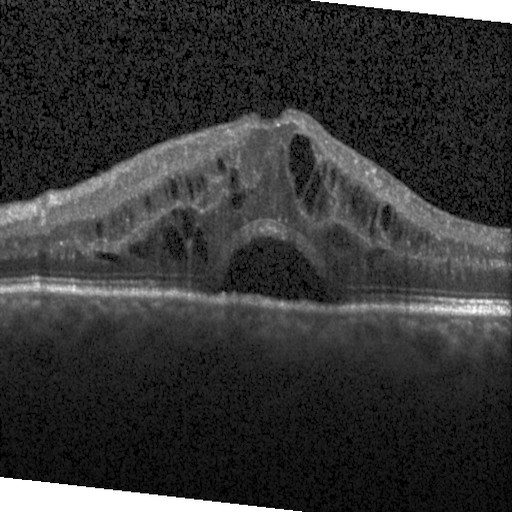
Spectral-domain OCT; OCT B-scan
This B-scan demonstrates DME.